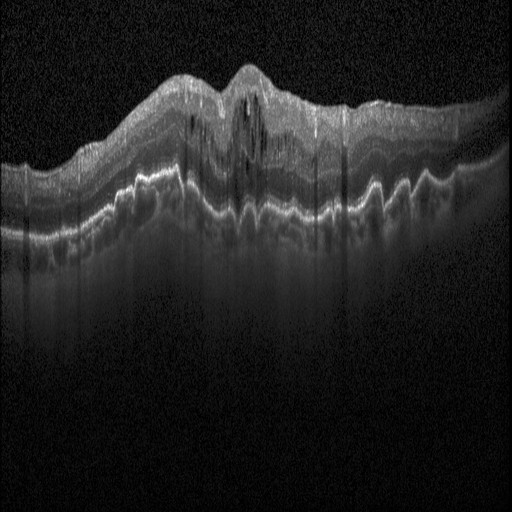

Macular scan; spectral-domain optical coherence tomography; Heidelberg Spectralis OCT system; retinal OCT B-scan.
Assessment: DME.